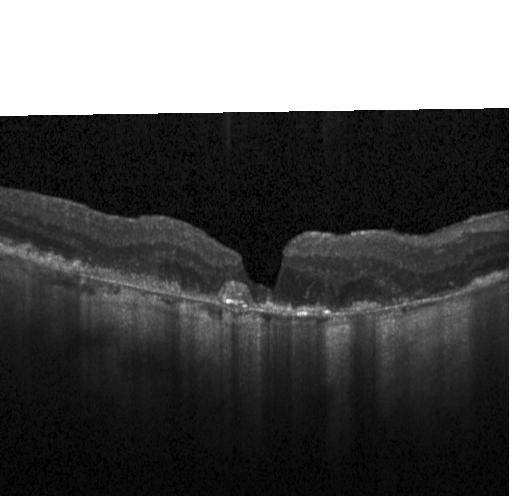 OCT B-scan showing choroidal neovascularization.